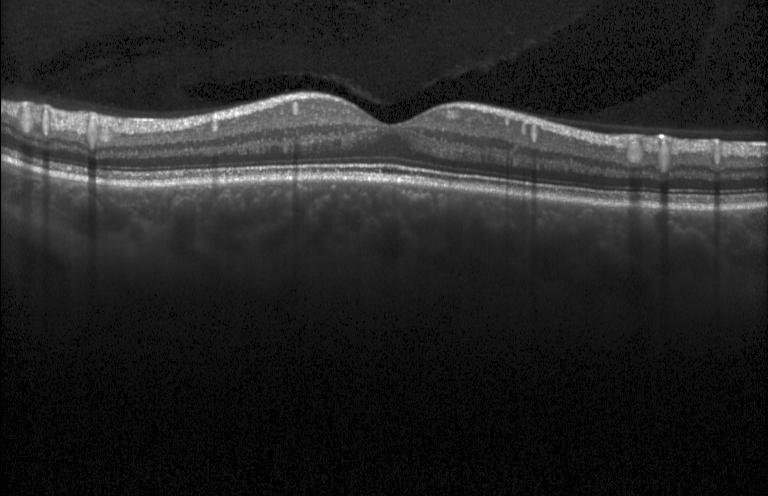

Impression: no choroidal neovascularization, no diabetic macular edema, and no drusen.